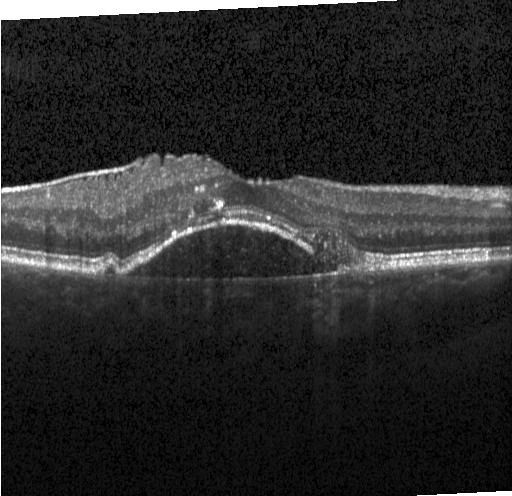
OCT B-scan
Choroidal neovascularization.